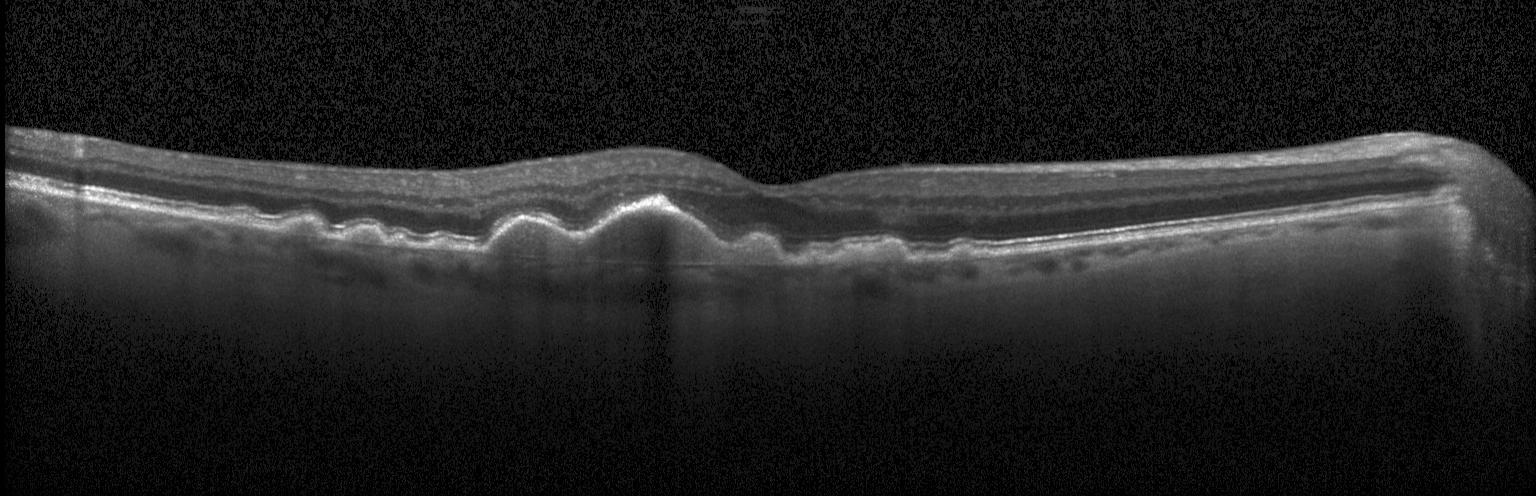

Impression: CNV.